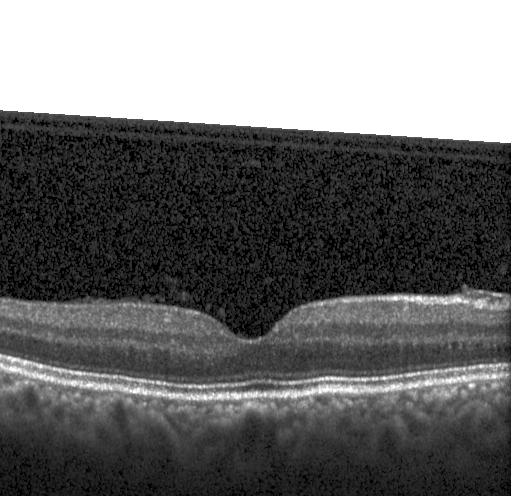
Optical coherence tomography scan; spectral-domain optical coherence tomography. Dx: no evidence of choroidal neovascularization, diabetic macular edema, or drusen.